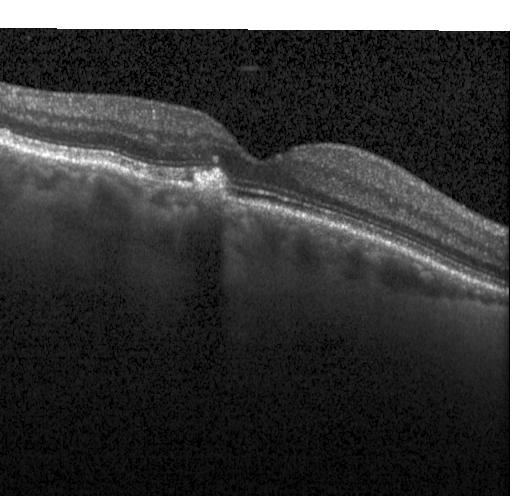
Finding: multiple drusen.